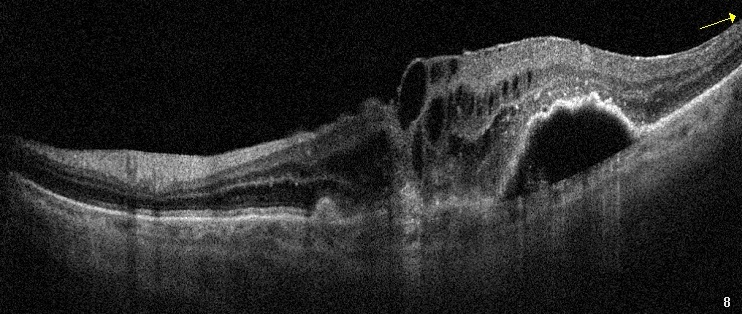
Fovea-centered; instrument: Optovue Avanti RTVue XR; optical coherence tomography B-scan.
Impression: AMD.